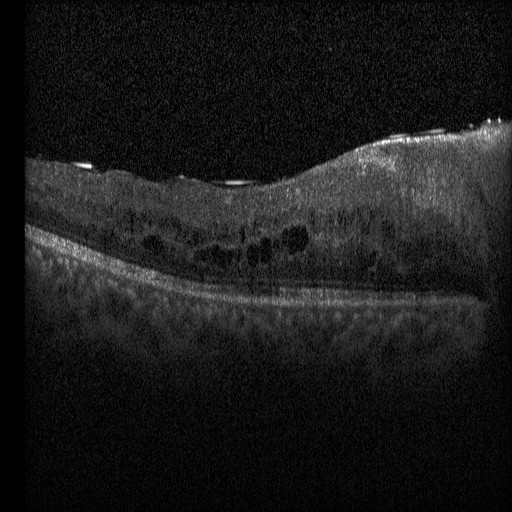

This B-scan demonstrates diabetic macular edema (DME).